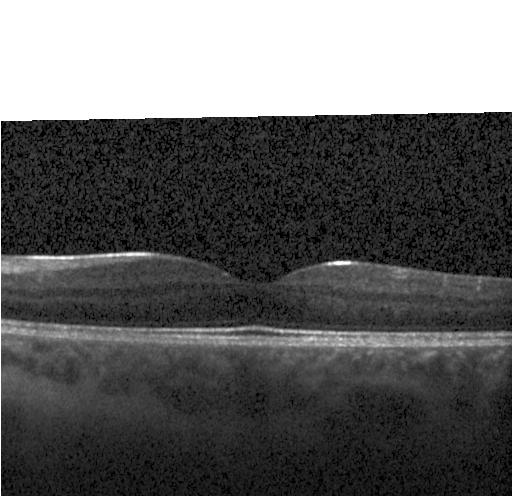

Optical coherence tomography B-scan; Heidelberg Spectralis OCT system — Assessment: neither CNV, DME, nor drusen.